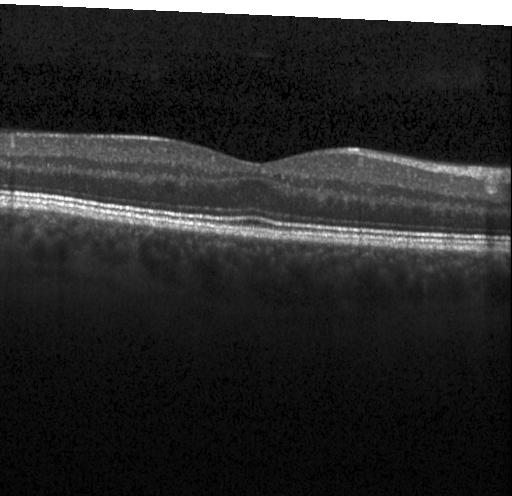

OCT B-scan — Macular OCT: neither choroidal neovascularization, diabetic macular edema, nor drusen.